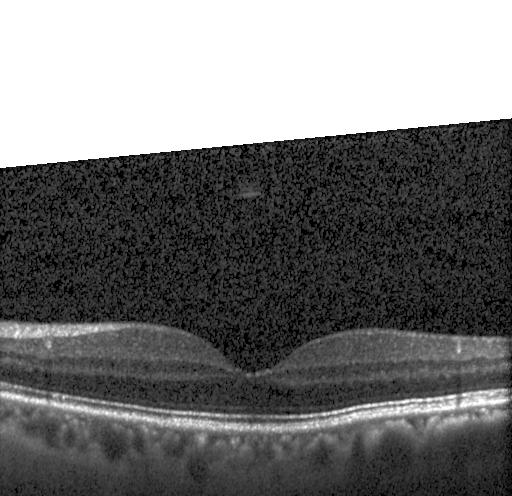

Horizontal scan through the fovea, spectral-domain optical coherence tomography, retinal OCT B-scan. Diagnosis: no evidence of choroidal neovascularization, diabetic macular edema, or drusen.